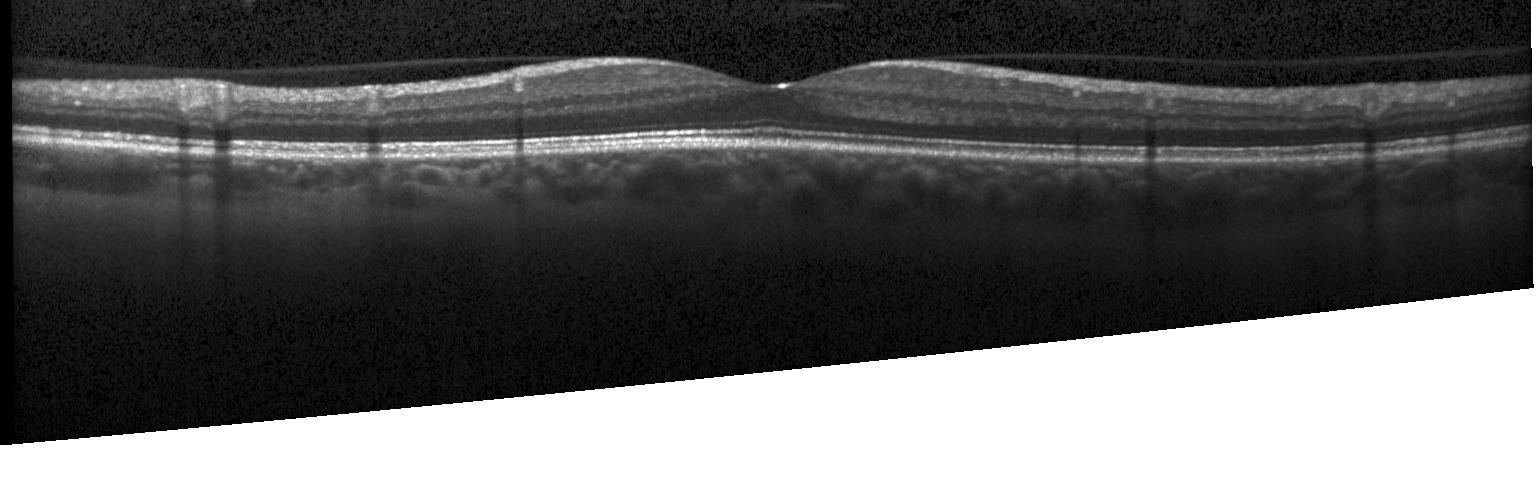

Assessment: no CNV, no DME, and no drusen.